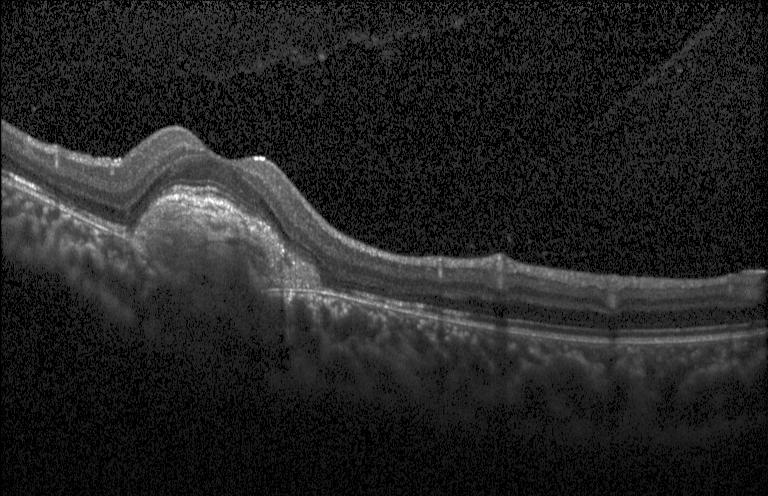 Spectral-domain optical coherence tomography, macular scan, OCT B-scan, Heidelberg Spectralis.
The scan shows a choroidal neovascular membrane.